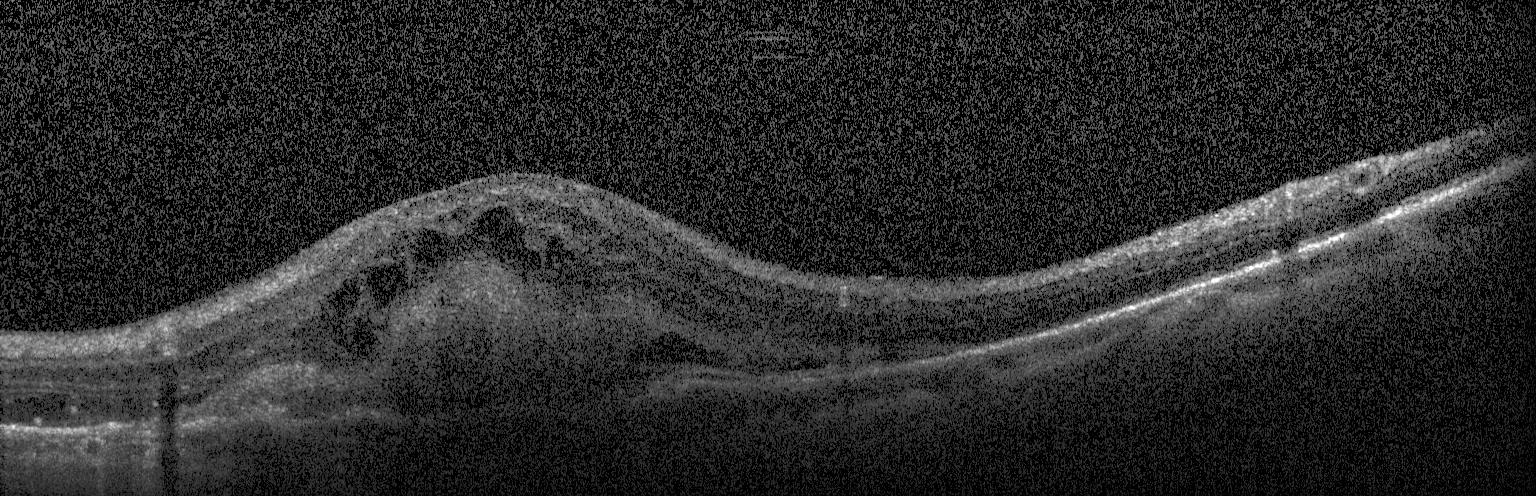

Acquired on a Heidelberg Spectralis, retinal OCT B-scan, through the macula.
Impression: a choroidal neovascular membrane.